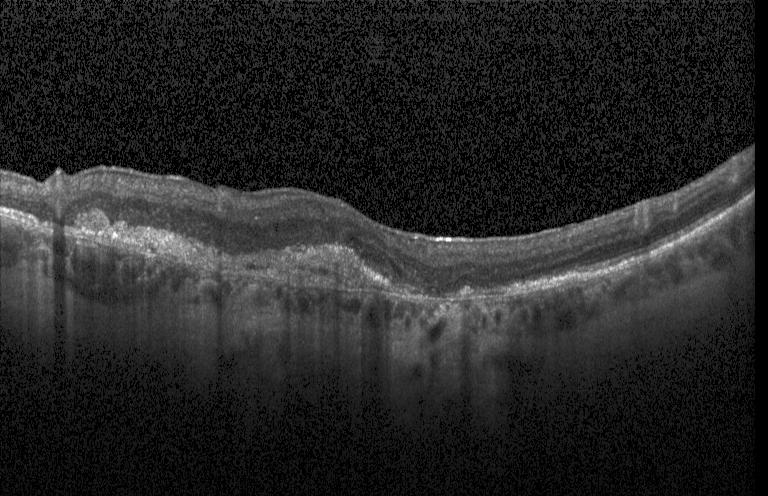

The scan shows a choroidal neovascular membrane.